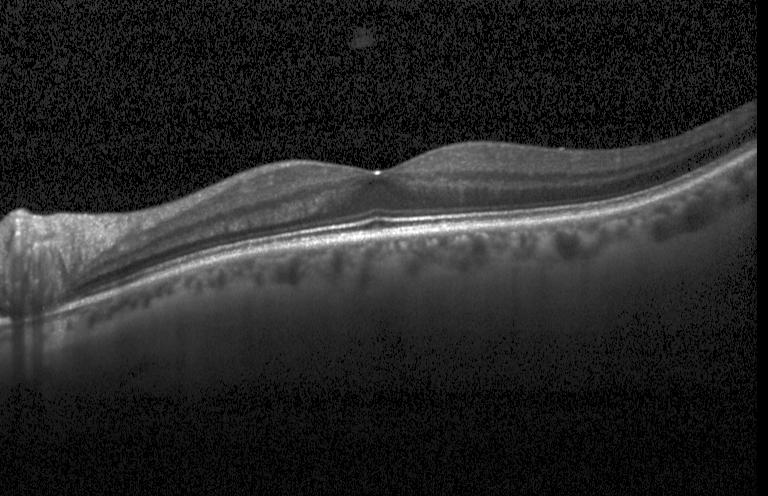
Centered on the fovea · Heidelberg Spectralis OCT system · optical coherence tomography scan
Assessment: no choroidal neovascularization, no diabetic macular edema, and no drusen.